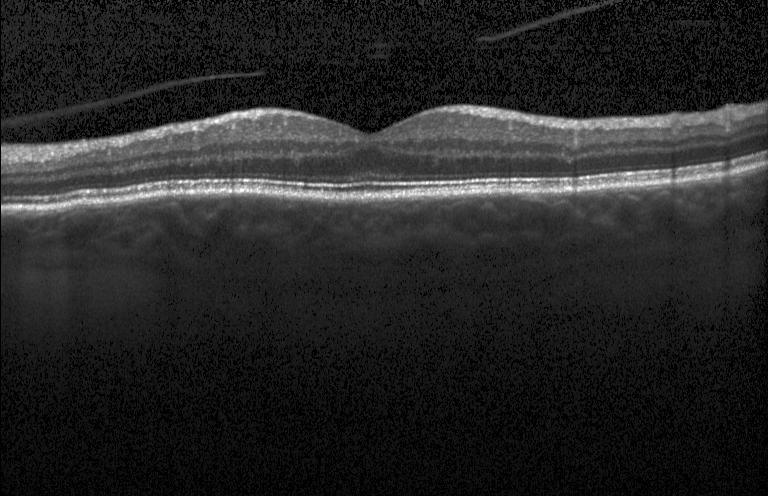

OCT B-scan; spectral-domain OCT
Diagnosis: no CNV, no DME, and no drusen.